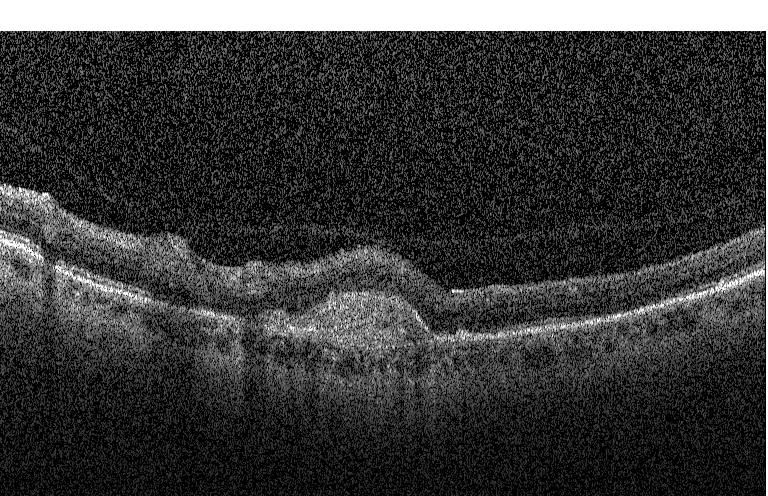
OCT B-scan. SD-OCT.
Dx: a choroidal neovascular membrane.